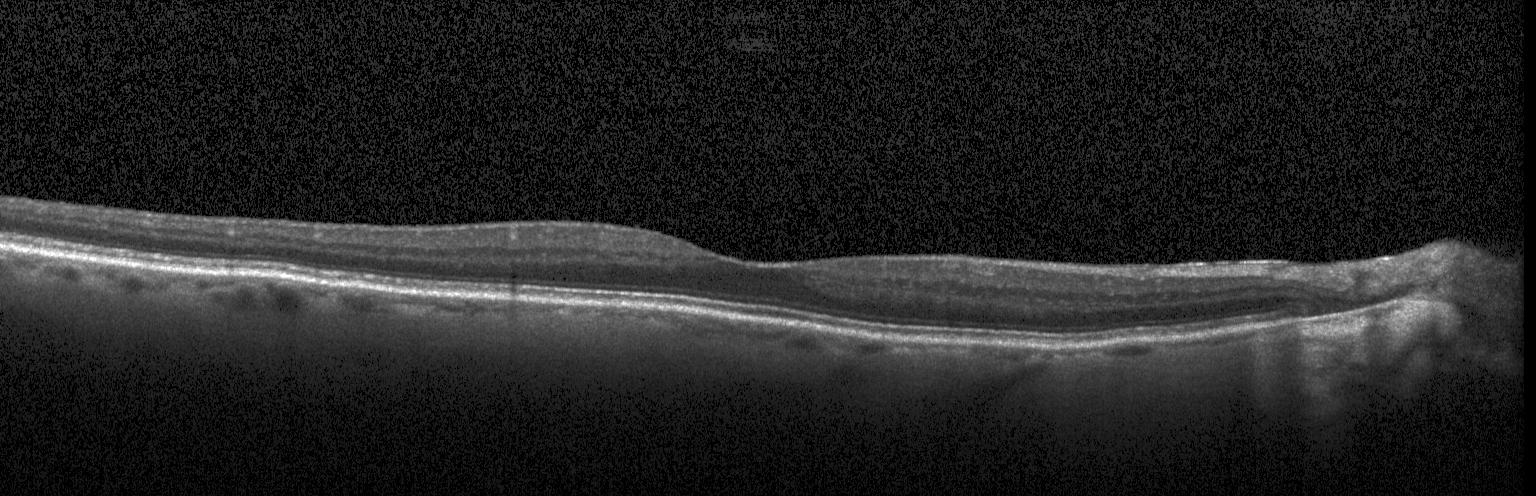 OCT finding: no CNV, DME, or drusen.